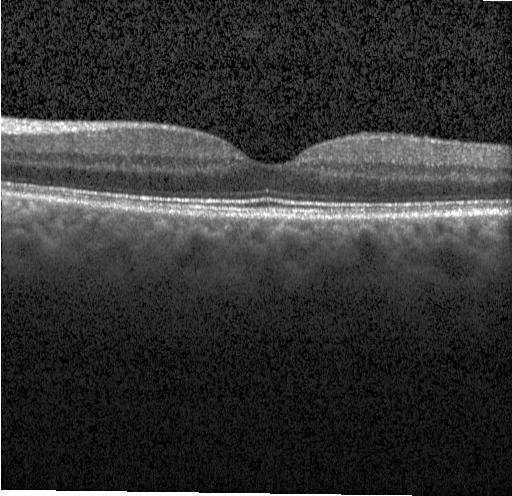 OCT B-scan showing no evidence of choroidal neovascularization, diabetic macular edema, or drusen.